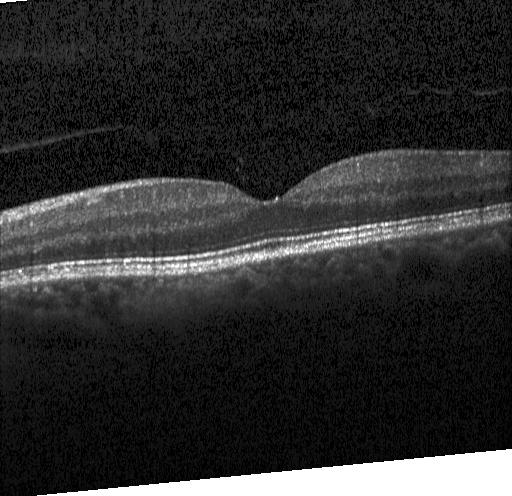 Heidelberg Spectralis OCT system. SD-OCT. OCT line scan.
Diagnosis: no choroidal neovascularization, diabetic macular edema, or drusen.